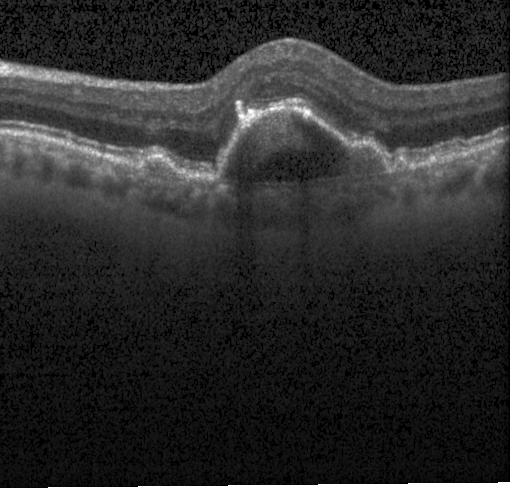

Retinal OCT cross-section showing sub-RPE drusenoid deposits.